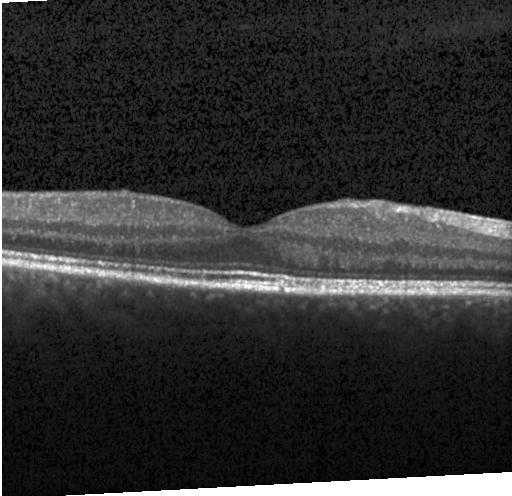
OCT finding: no choroidal neovascularization, no diabetic macular edema, and no drusen.